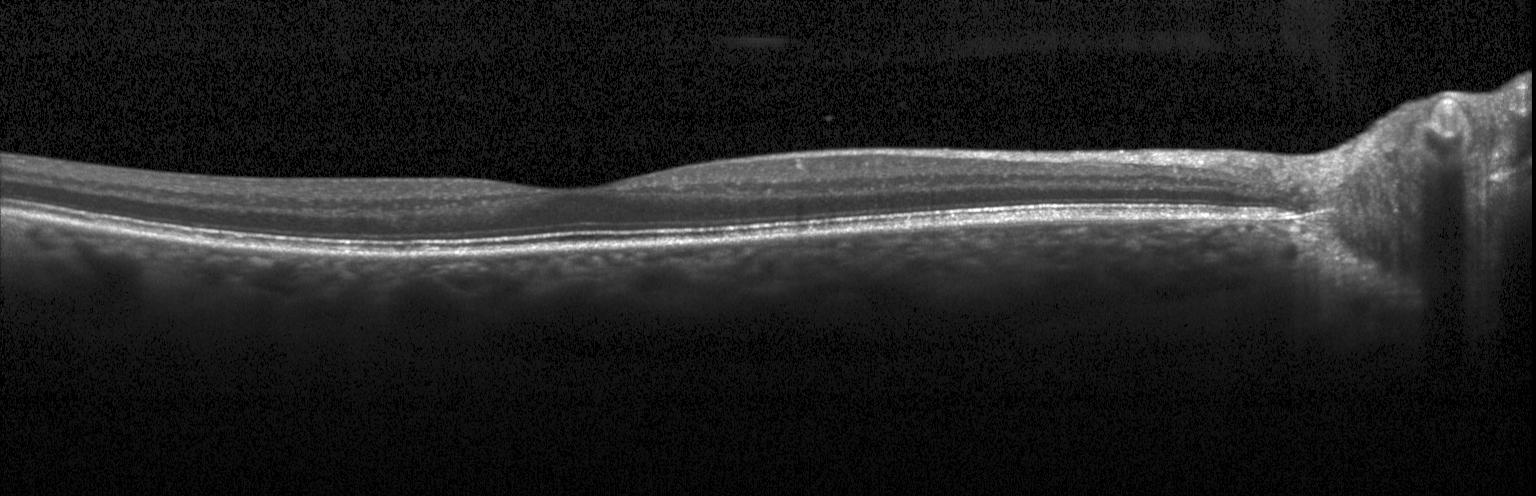

Retinal OCT cross-section
Impression: no CNV, DME, or drusen.